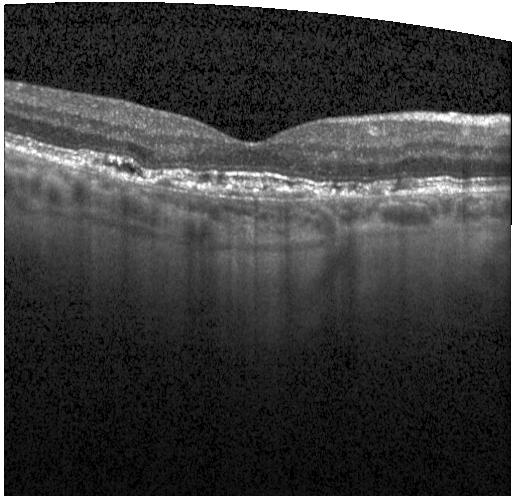
OCT B-scan — CNV.